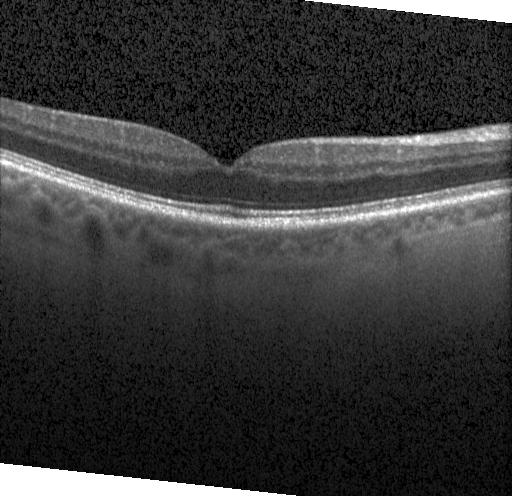 Heidelberg Spectralis · retinal OCT B-scan — The scan shows neither choroidal neovascularization, diabetic macular edema, nor drusen.